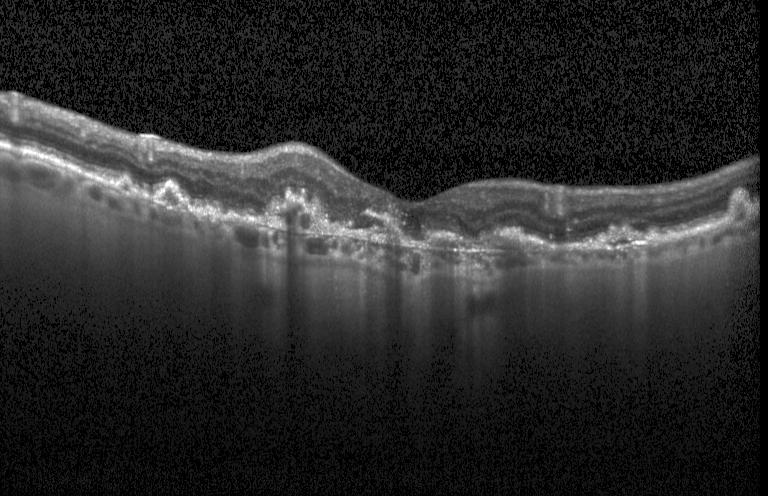 Through the macula, OCT B-scan, instrument: Heidelberg Spectralis, spectral-domain OCT. Finding: choroidal neovascularization (CNV).